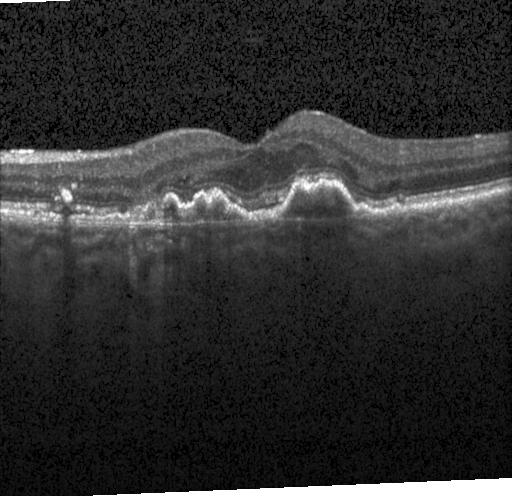
Diagnosis: a choroidal neovascular membrane.